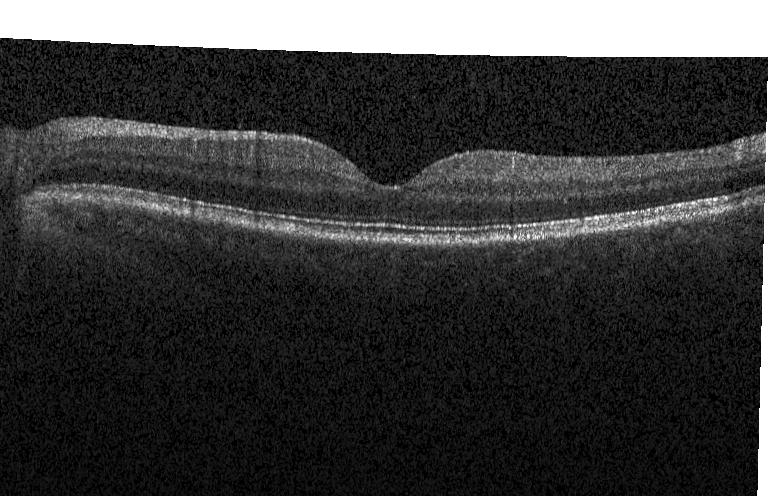

Optical coherence tomography B-scan
Diagnosis: no evidence of choroidal neovascularization, diabetic macular edema, or drusen.